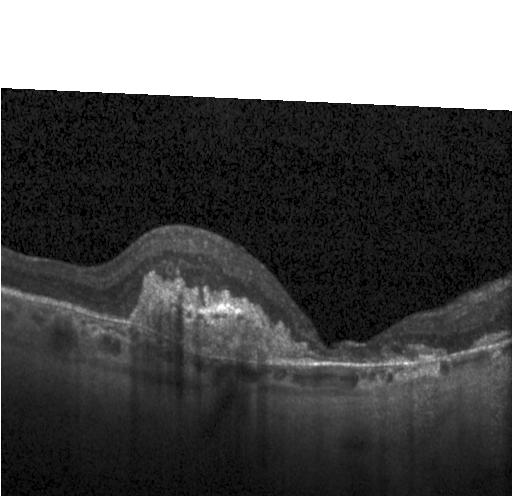

Retinal OCT cross-section. Spectral-domain OCT.
Impression: choroidal neovascularization (CNV).